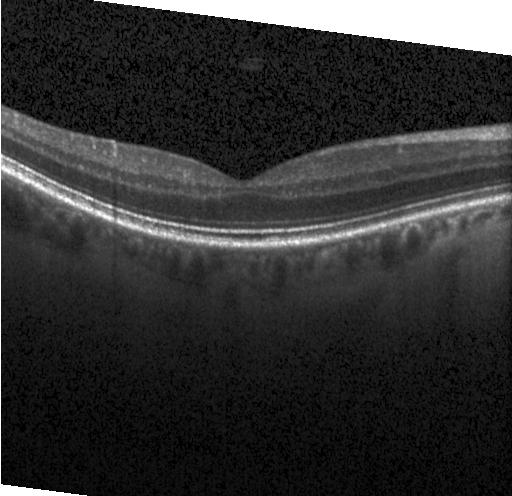 Through the macula; retinal OCT B-scan. Diagnosis: no evidence of CNV, DME, or drusen.